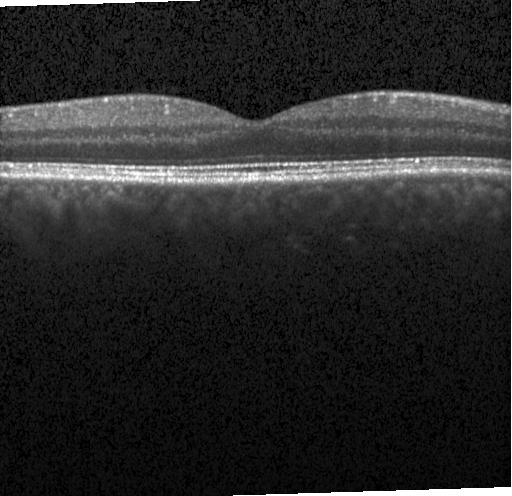
OCT B-scan. Acquired on a Heidelberg Spectralis. Horizontal scan through the fovea. Spectral-domain OCT — No evidence of choroidal neovascularization, diabetic macular edema, or drusen.